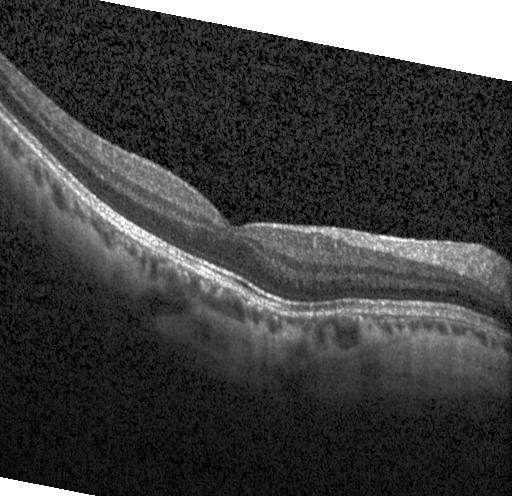

OCT B-scan, macular scan
Macular OCT: neither choroidal neovascularization, diabetic macular edema, nor drusen.